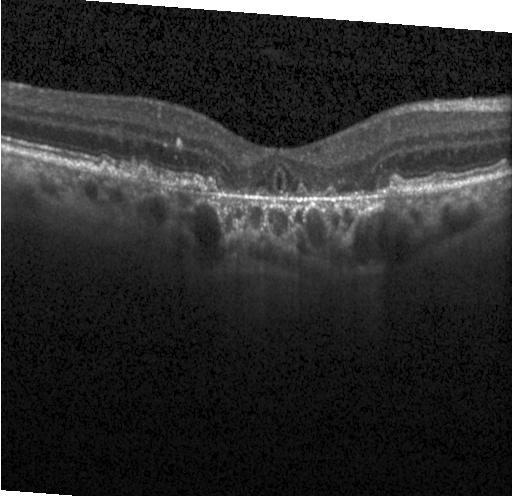

Macular OCT: choroidal neovascularization.